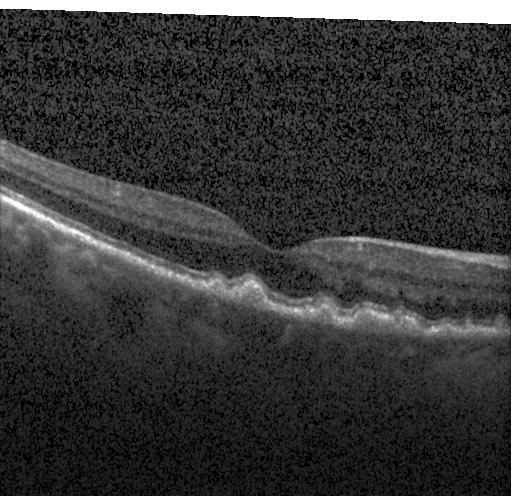 Centered on the fovea; retinal OCT cross-section; spectral-domain OCT — Diagnosis: sub-RPE drusenoid deposits.